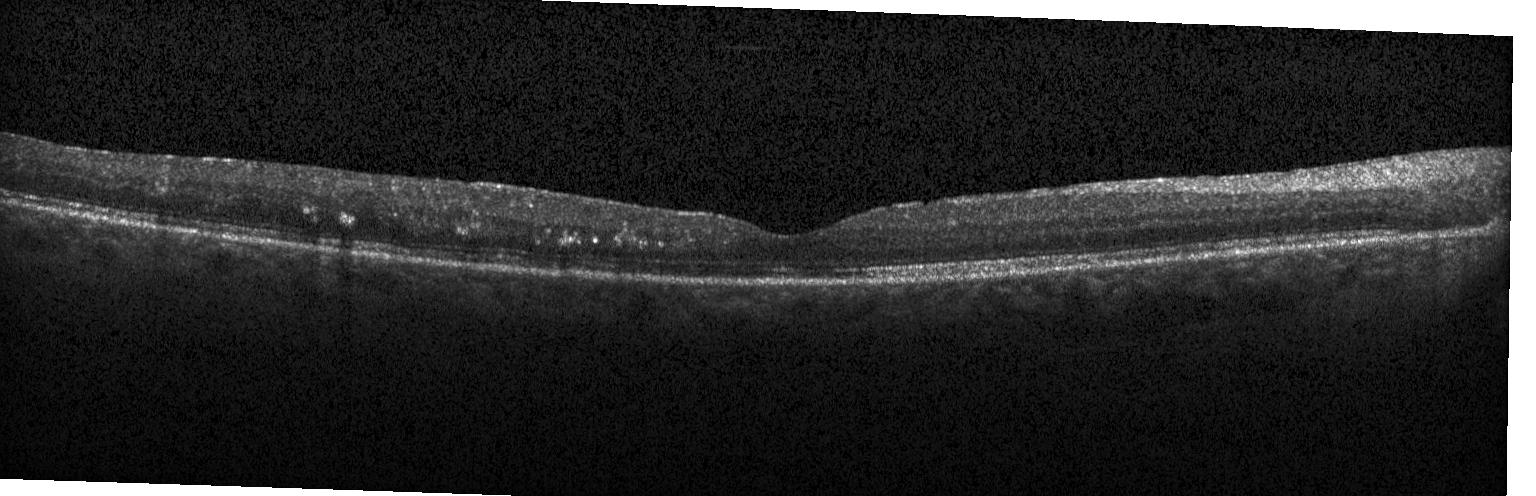 Heidelberg Spectralis; spectral-domain OCT; retinal OCT B-scan; fovea-centered
Finding: diabetic macular edema (DME).